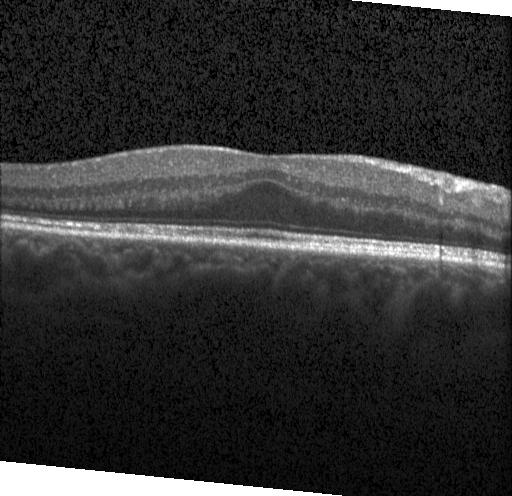 OCT line scan. SD-OCT — Diagnosis: no CNV, no DME, and no drusen.